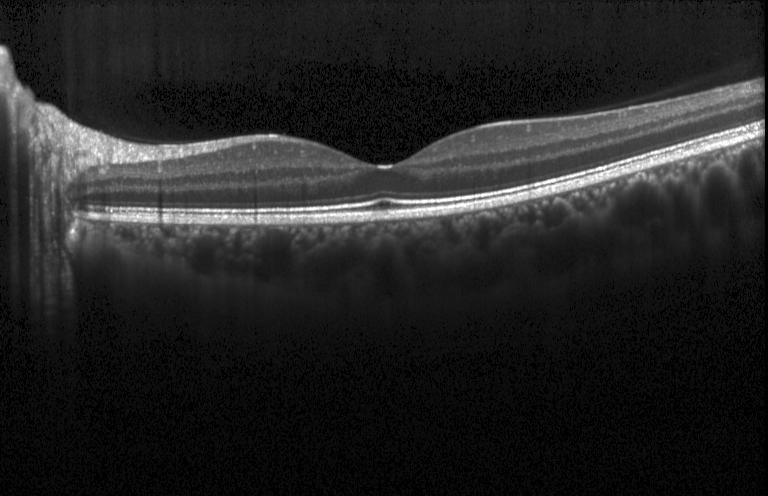 Retinal OCT cross-section showing no CNV, no DME, and no drusen.